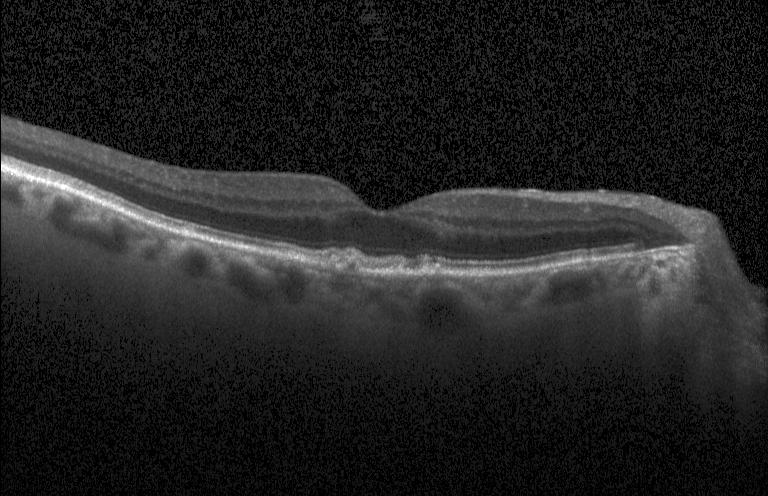 OCT line scan. The scan shows sub-RPE drusenoid deposits.